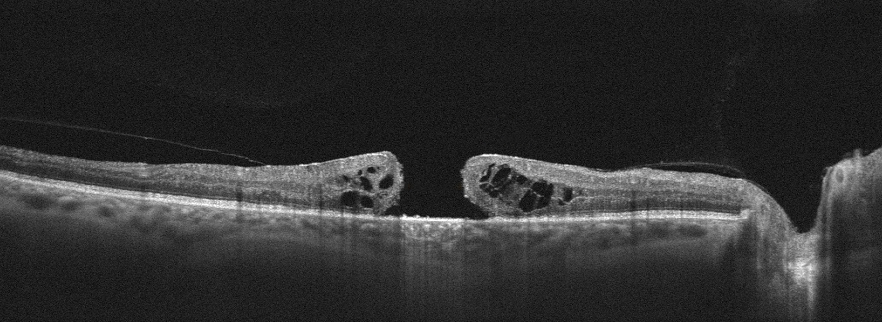

OCT B-scan. Oculus dexter
Macular OCT: VID.